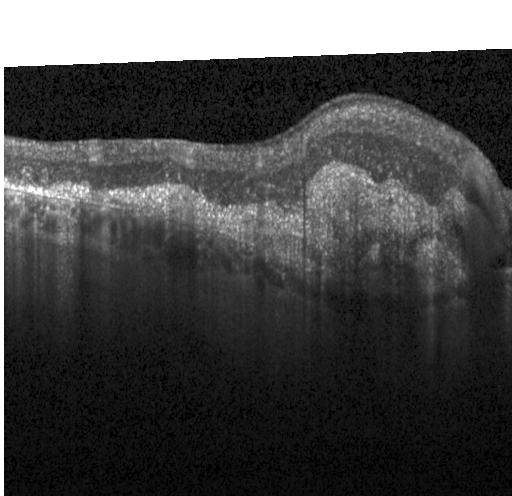
Retinal OCT cross-section, fovea-centered, SD-OCT. Diagnosis: a choroidal neovascular membrane.